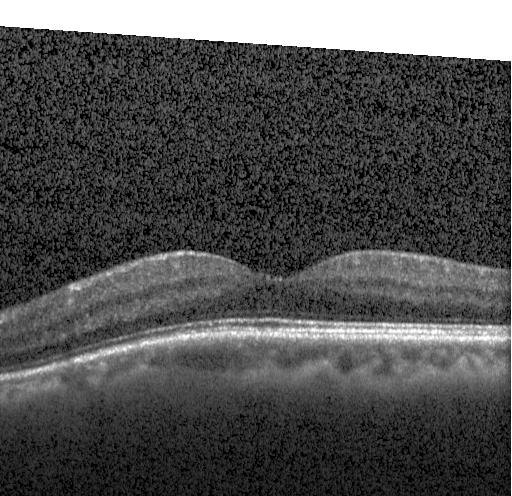
Spectral-domain OCT · instrument: Heidelberg Spectralis · optical coherence tomography scan · through the macula — This B-scan demonstrates no choroidal neovascularization, diabetic macular edema, or drusen.